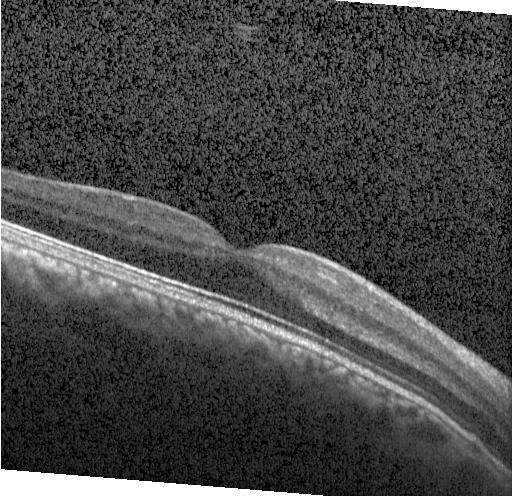

The scan shows neither choroidal neovascularization, diabetic macular edema, nor drusen.